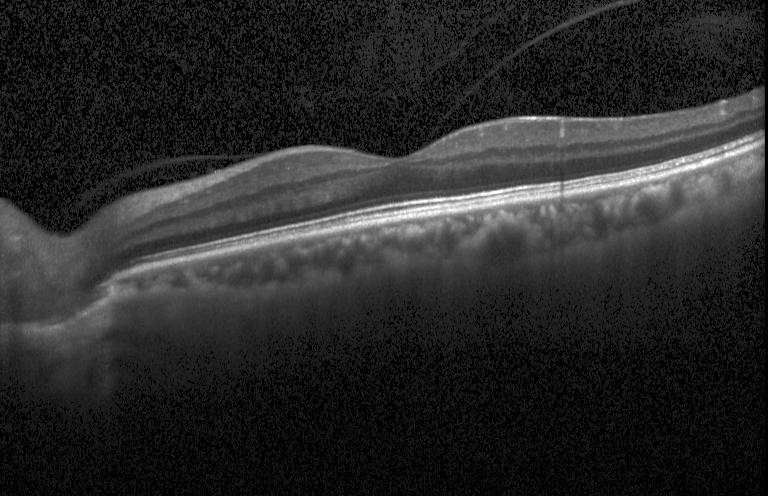 Fovea-centered · OCT line scan — The scan shows no choroidal neovascularization, no diabetic macular edema, and no drusen.